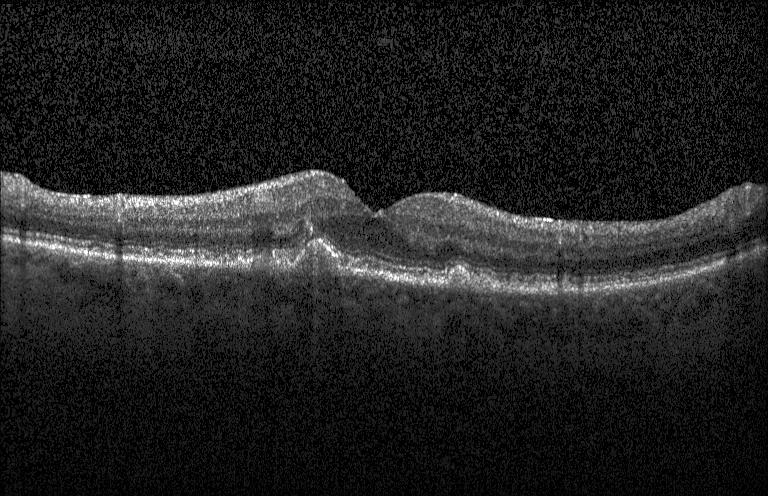

Retinal OCT cross-section · centered on the fovea — OCT finding: multiple drusen.